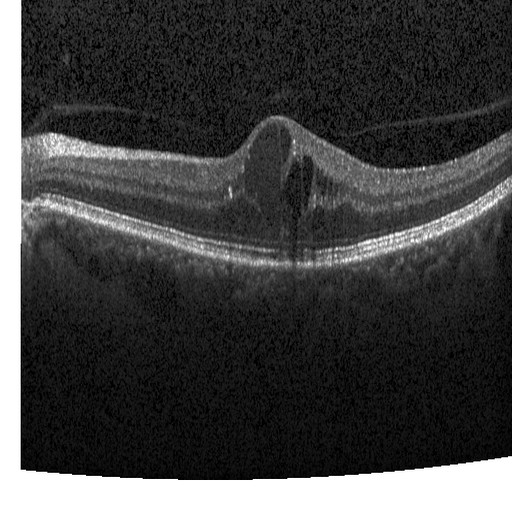

OCT scan showing diabetic macular edema (DME).